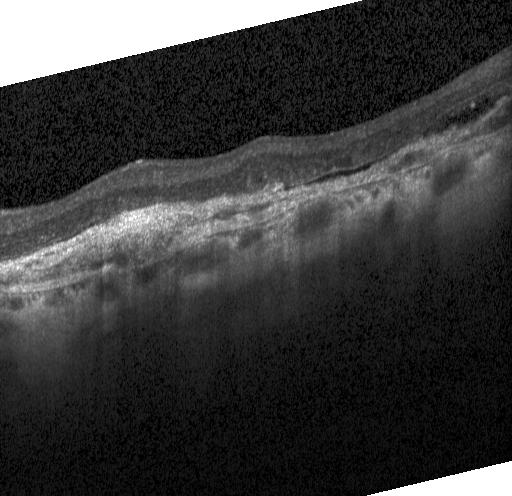
Retinal OCT cross-section, Heidelberg Spectralis OCT system, spectral-domain optical coherence tomography, horizontal scan through the fovea
Impression: a choroidal neovascular membrane.